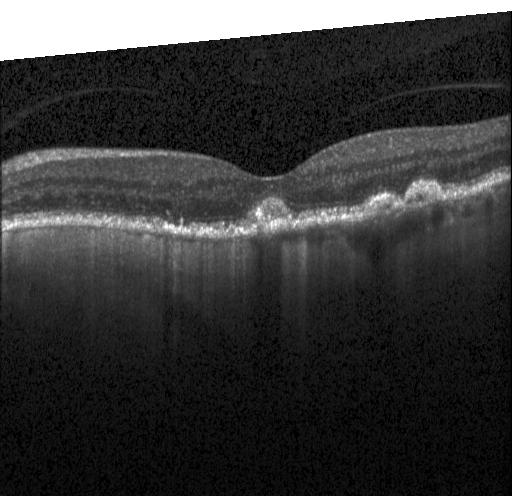 Macular OCT demonstrating drusen.